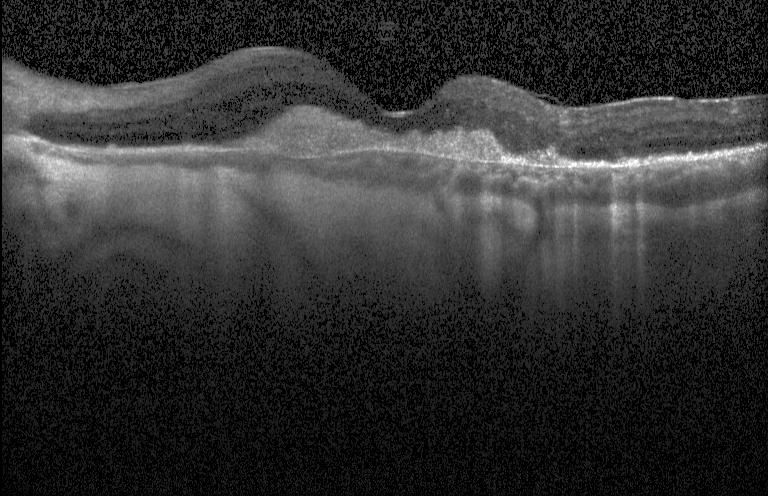

Retinal OCT B-scan
Dx: CNV.